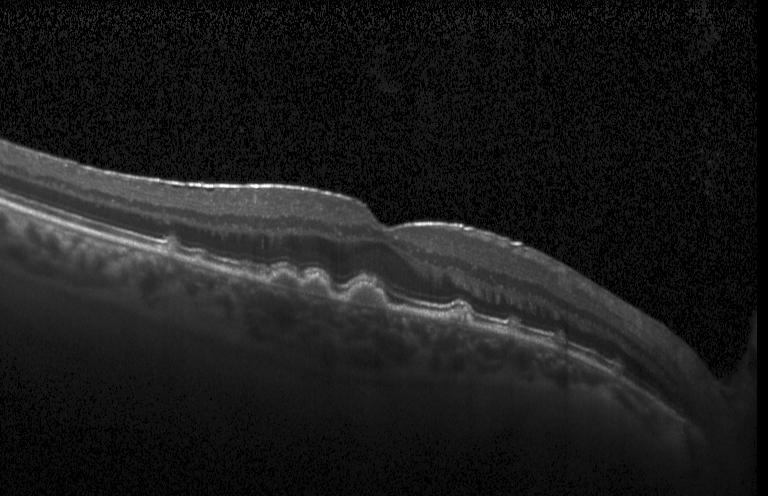
Instrument: Heidelberg Spectralis; retinal OCT cross-section.
This B-scan demonstrates multiple drusen.